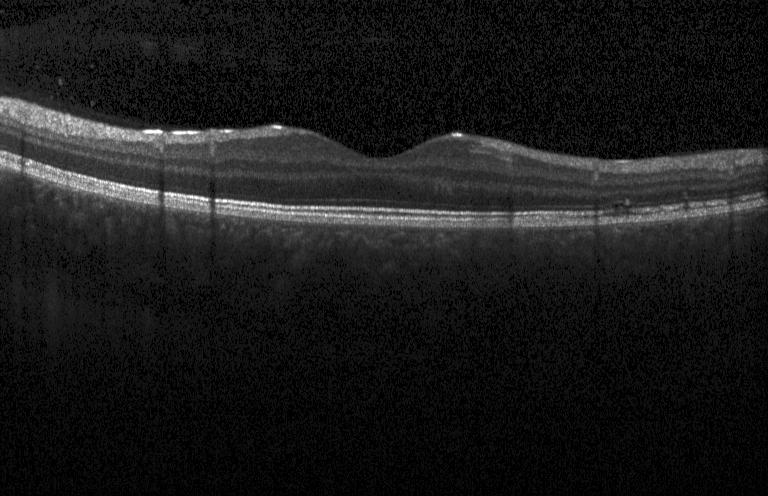
Dx: neither choroidal neovascularization, diabetic macular edema, nor drusen.